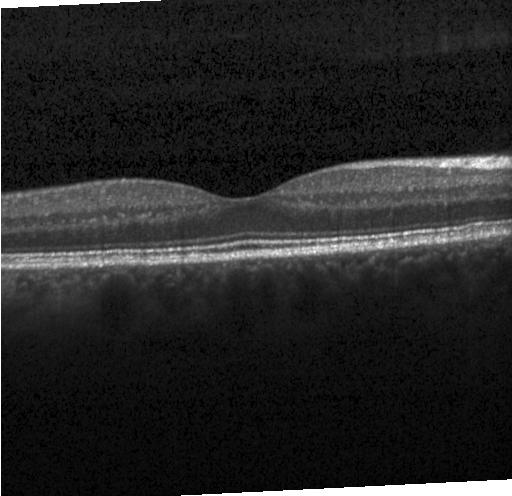
OCT finding: neither CNV, DME, nor drusen.